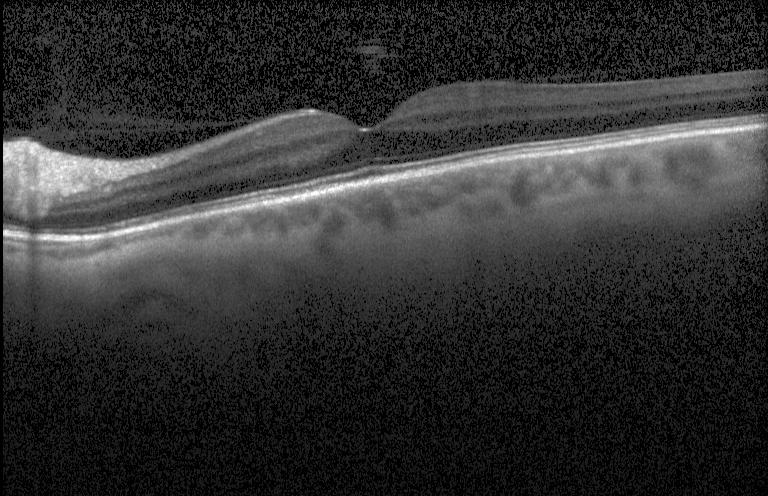 Impression: no evidence of choroidal neovascularization, diabetic macular edema, or drusen.